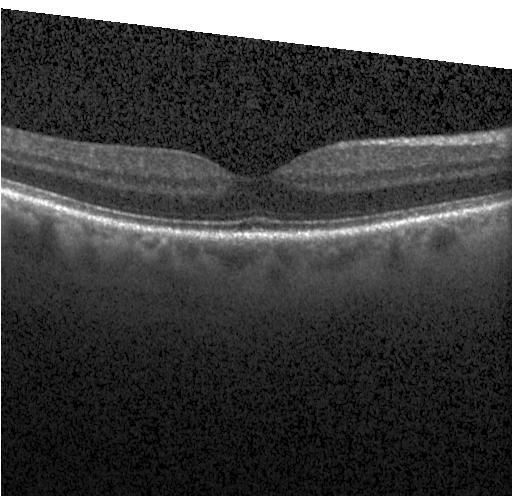

Acquired on a Heidelberg Spectralis, optical coherence tomography B-scan
Macular OCT: no CNV, DME, or drusen.